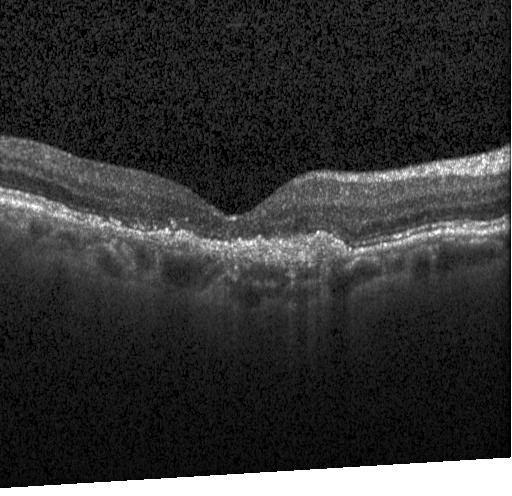

Heidelberg Spectralis OCT system. OCT B-scan. Centered on the fovea. SD-OCT. Choroidal neovascularization (CNV).